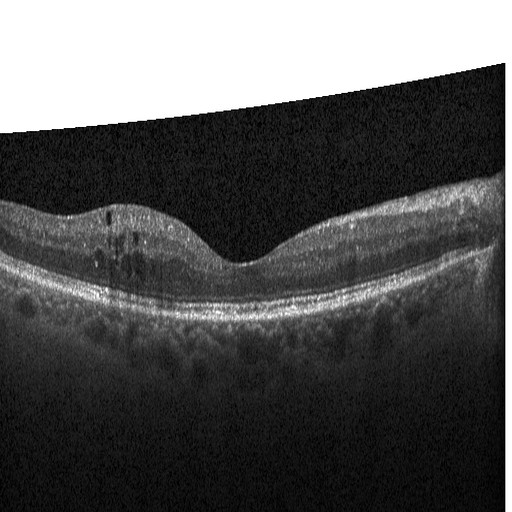 Diagnosis: diabetic macular edema.